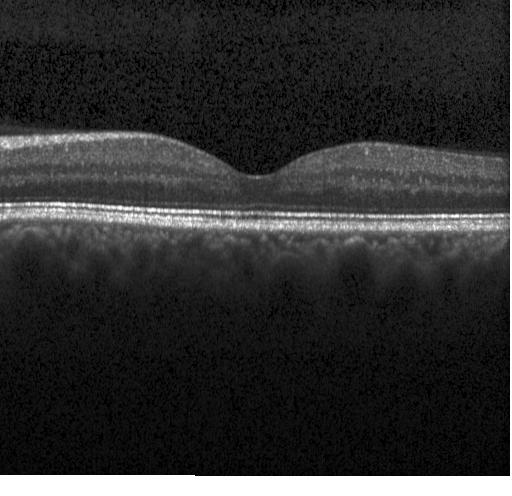

Spectral-domain OCT, Heidelberg Spectralis, optical coherence tomography B-scan
No choroidal neovascularization, diabetic macular edema, or drusen.